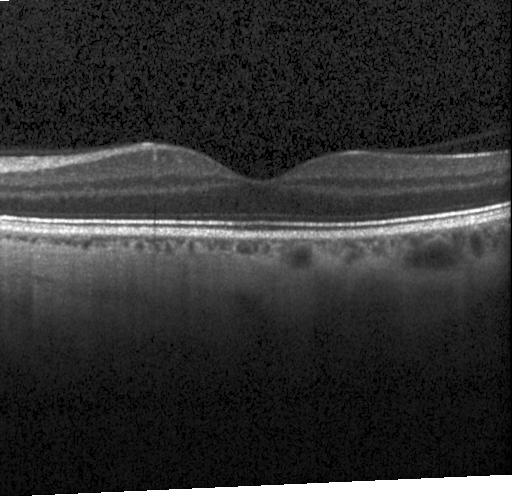
Spectral-domain OCT · centered on the fovea · acquired on a Heidelberg Spectralis · optical coherence tomography B-scan.
Assessment: no evidence of choroidal neovascularization, diabetic macular edema, or drusen.